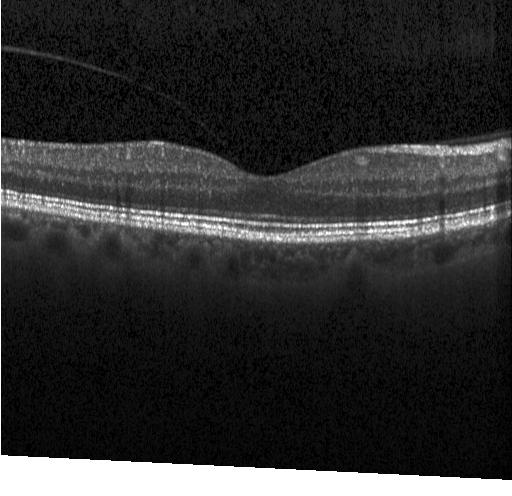
Impression: no evidence of CNV, DME, or drusen.